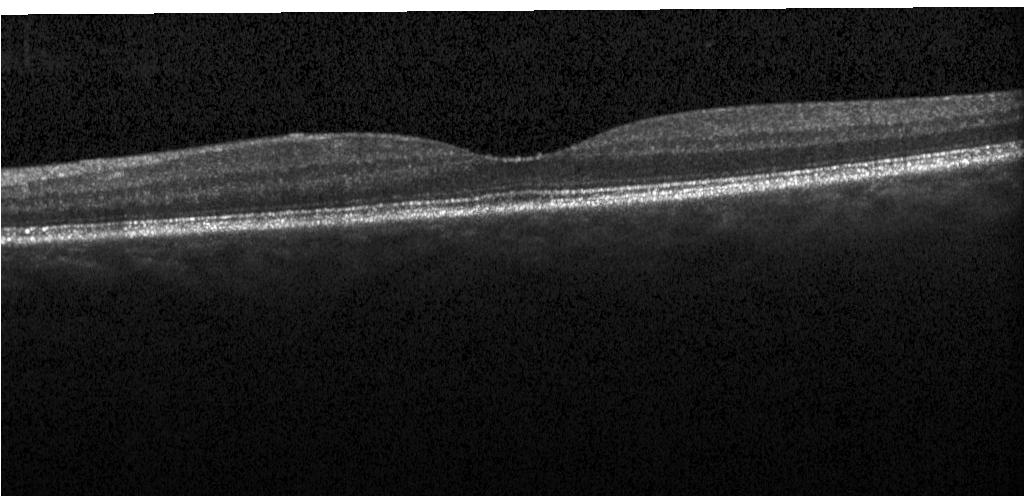
Retinal OCT cross-section — No evidence of CNV, DME, or drusen.